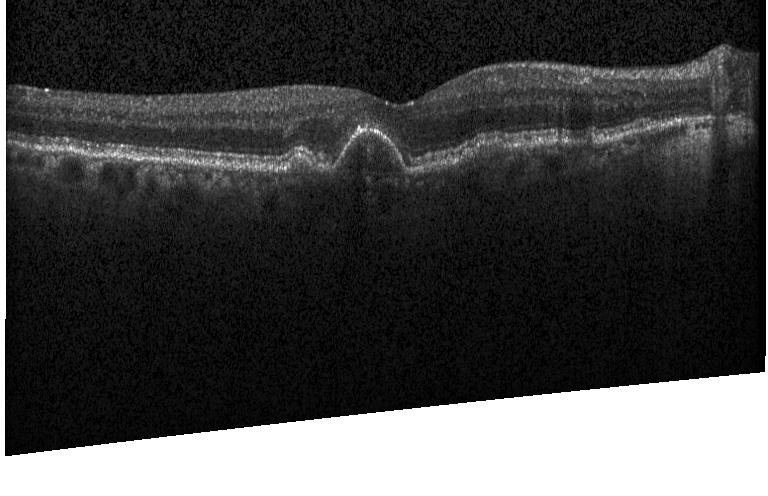
Heidelberg Spectralis OCT system, centered on the fovea, SD-OCT, retinal OCT cross-section — Diagnosis: multiple drusen.